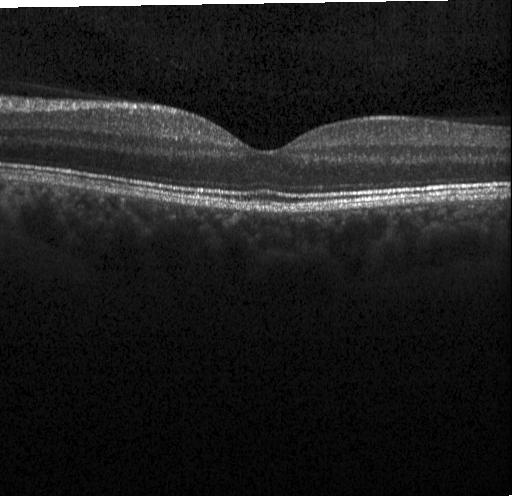 Macular OCT demonstrating no CNV, no DME, and no drusen.